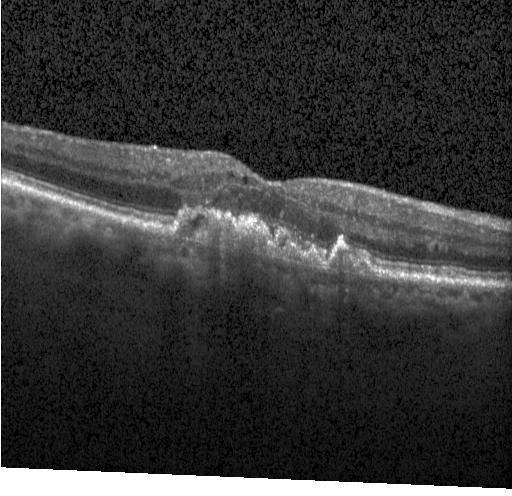 Choroidal neovascularization.